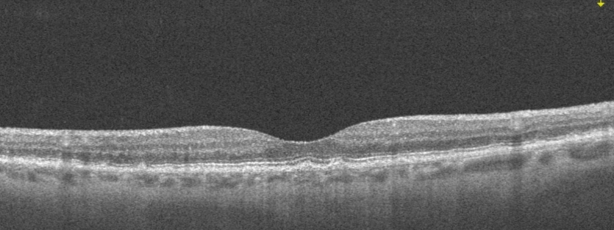

OCT B-scan, macular scan, Optovue Avanti RTVue XR.
Age-related macular degeneration (AMD).